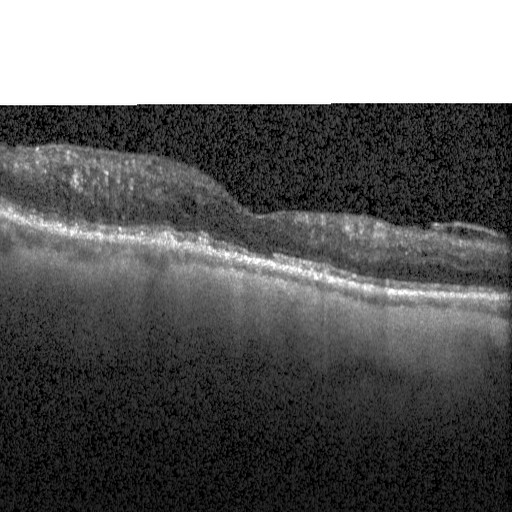 Diagnosis: diabetic macular edema (DME).